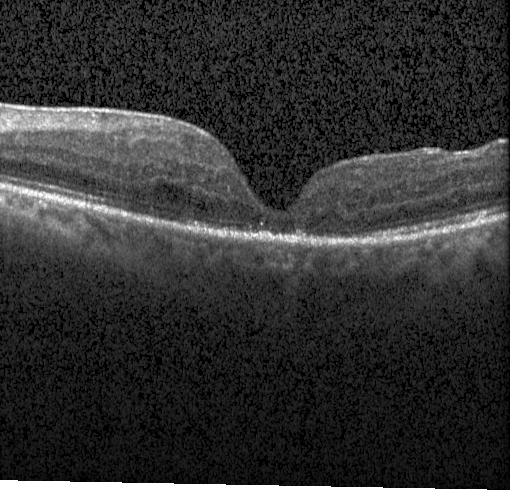

Retinal OCT B-scan. DME.